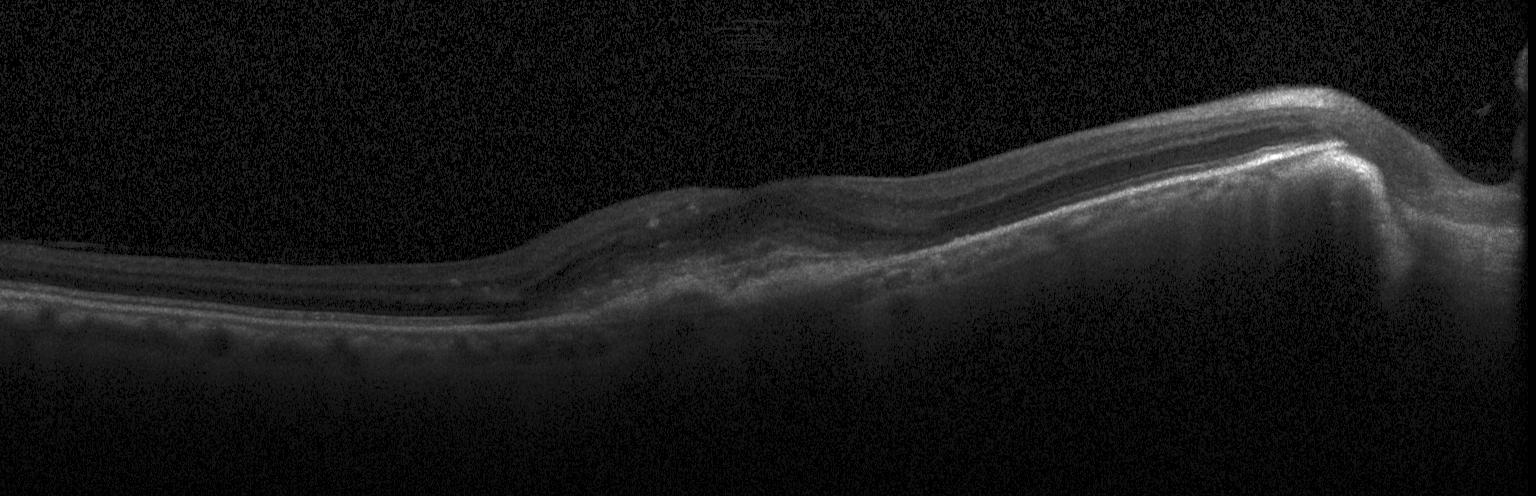
Optical coherence tomography scan. Spectral-domain OCT. Acquired on a Heidelberg Spectralis. Through the macula
This B-scan demonstrates CNV.